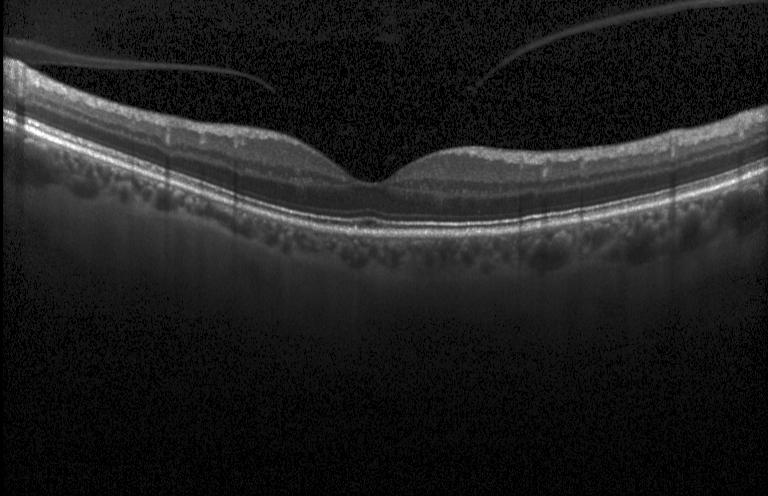
Finding: no choroidal neovascularization, diabetic macular edema, or drusen.